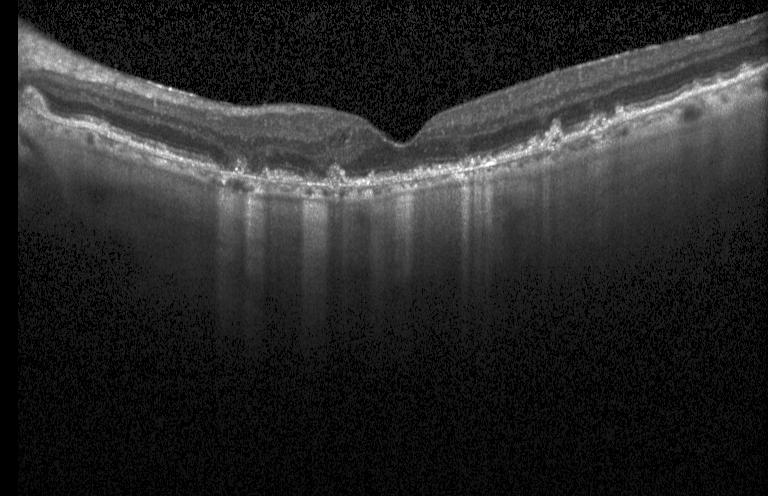

Heidelberg Spectralis OCT system. OCT line scan. CNV.